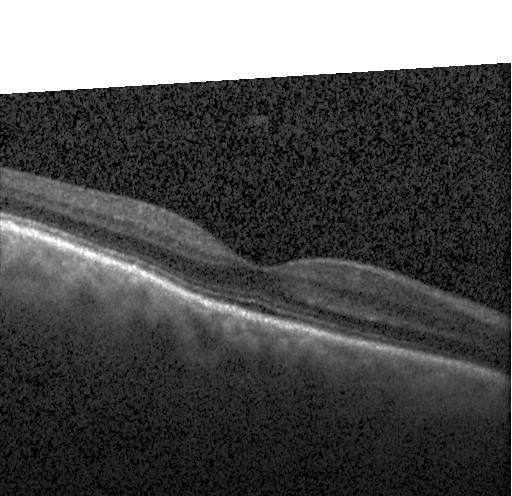 Heidelberg Spectralis, optical coherence tomography scan
Finding: no CNV, no DME, and no drusen.